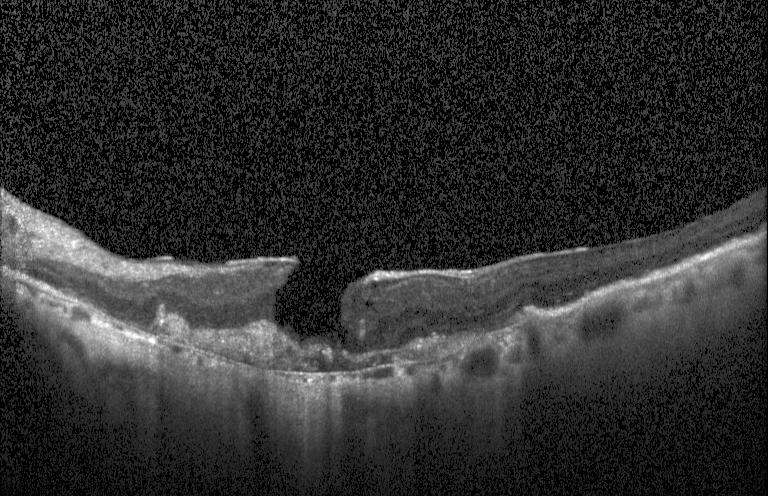 Heidelberg Spectralis OCT system; OCT B-scan — Diagnosis: choroidal neovascularization (CNV).